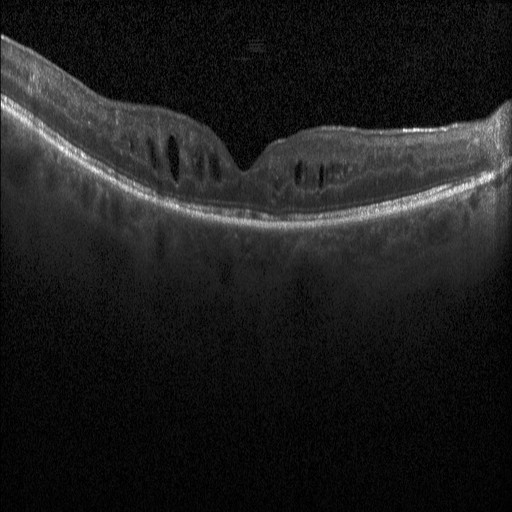

The scan shows diabetic macular edema.